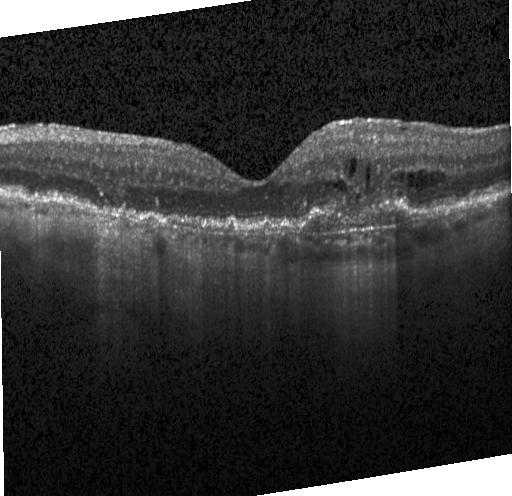

Impression: choroidal neovascularization.